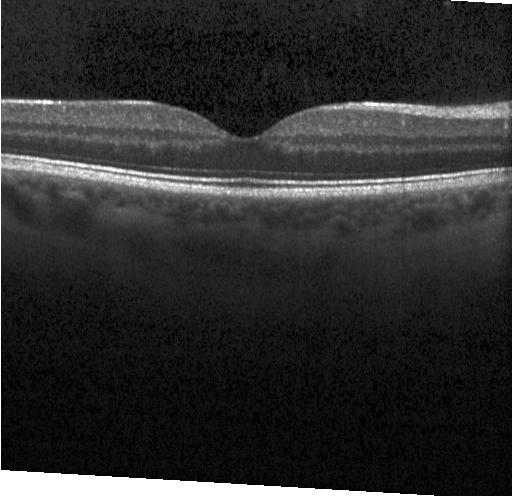 Optical coherence tomography B-scan.
Dx: no evidence of choroidal neovascularization, diabetic macular edema, or drusen.